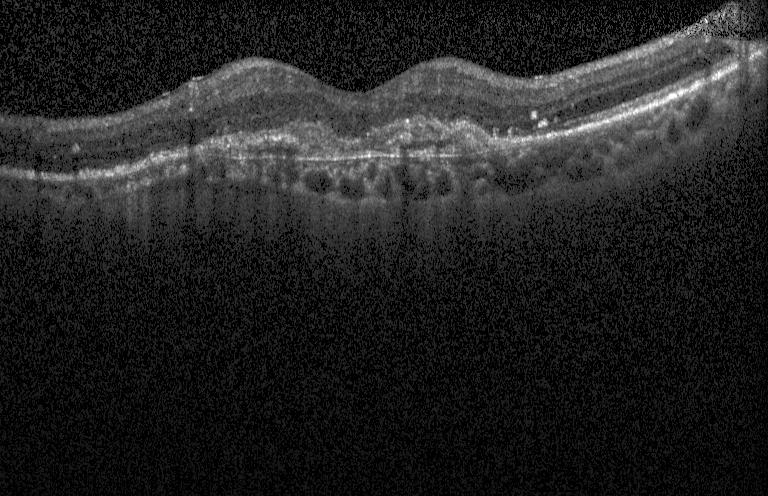

OCT B-scan
Macular OCT: choroidal neovascularization.